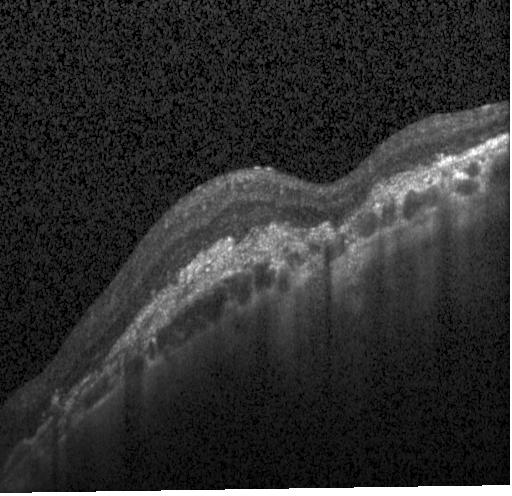 OCT B-scan showing choroidal neovascularization (CNV).